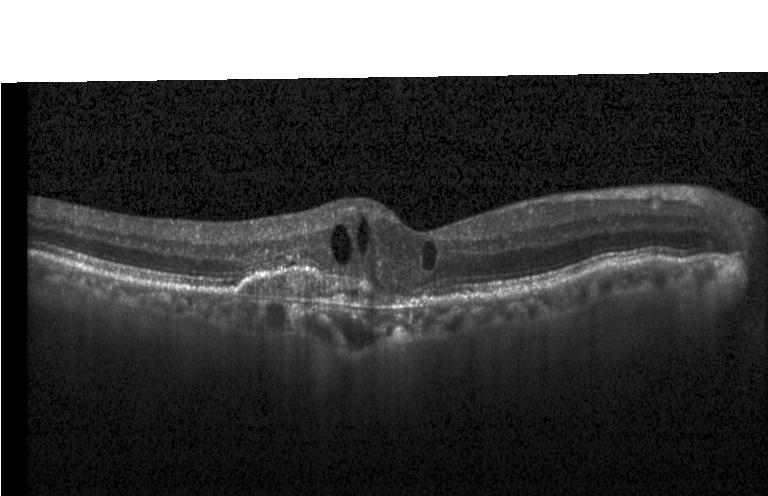 Spectral-domain OCT; OCT B-scan — OCT finding: a choroidal neovascular membrane.